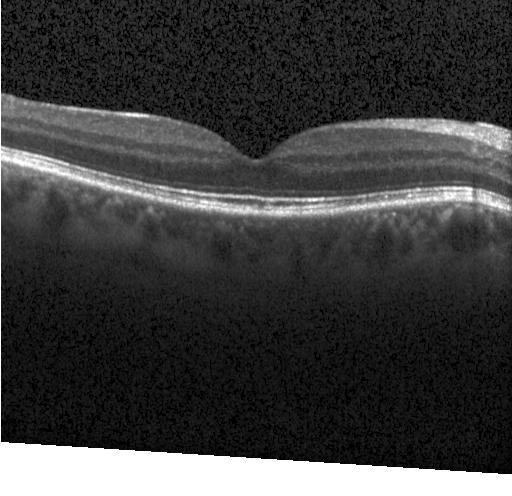

Optical coherence tomography scan.
Assessment: no evidence of choroidal neovascularization, diabetic macular edema, or drusen.